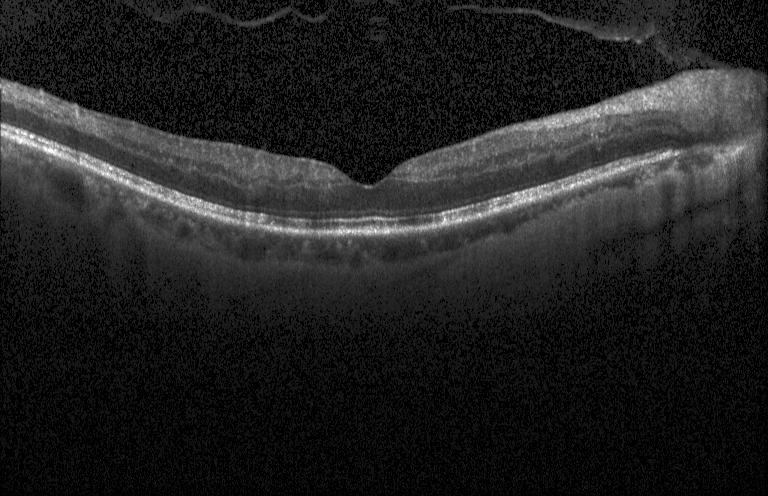

OCT B-scan. Impression: neither choroidal neovascularization, diabetic macular edema, nor drusen.